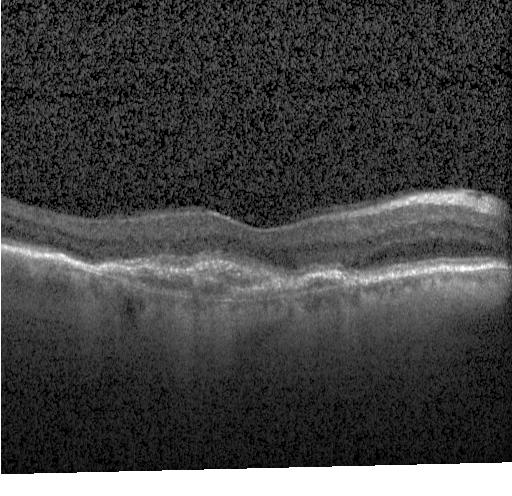
Impression: a choroidal neovascular membrane.